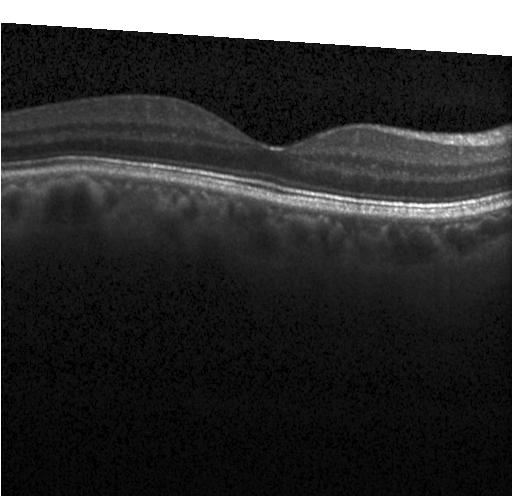

OCT scan showing no evidence of CNV, DME, or drusen.